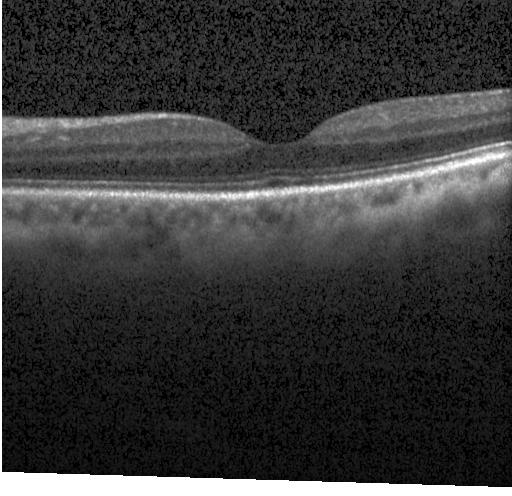 Spectral-domain optical coherence tomography; fovea-centered; optical coherence tomography scan — Macular OCT: neither choroidal neovascularization, diabetic macular edema, nor drusen.